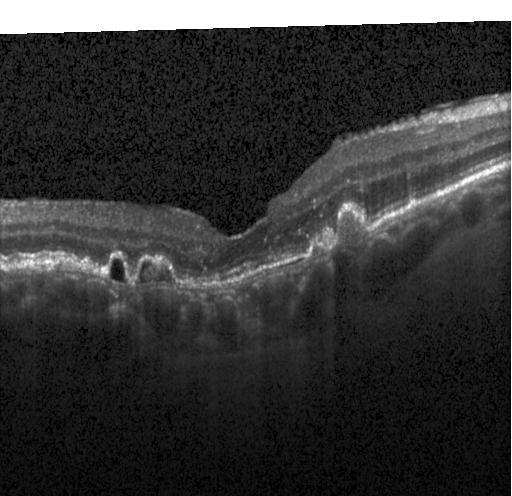 Retinal OCT B-scan · SD-OCT · macular scan
Impression: a choroidal neovascular membrane.